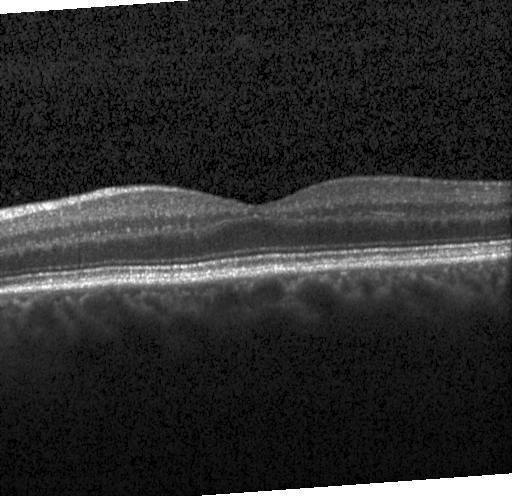 No evidence of CNV, DME, or drusen.